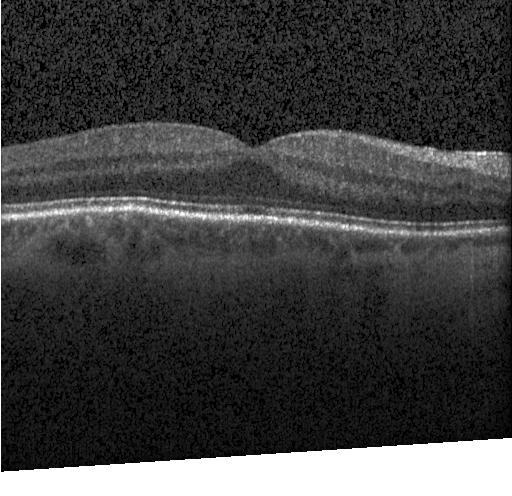
Spectral-domain optical coherence tomography, centered on the fovea, OCT B-scan. Finding: neither choroidal neovascularization, diabetic macular edema, nor drusen.